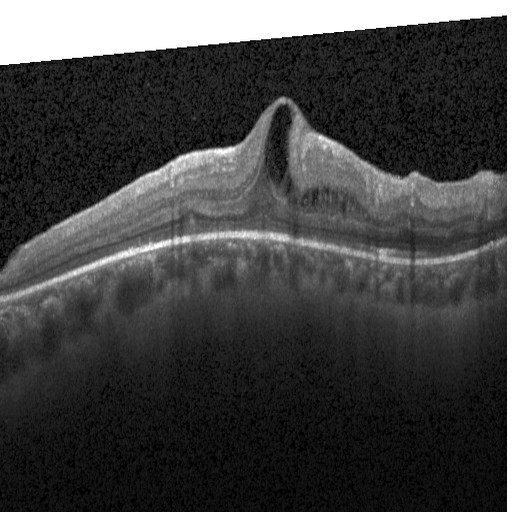

Macular OCT demonstrating DME.